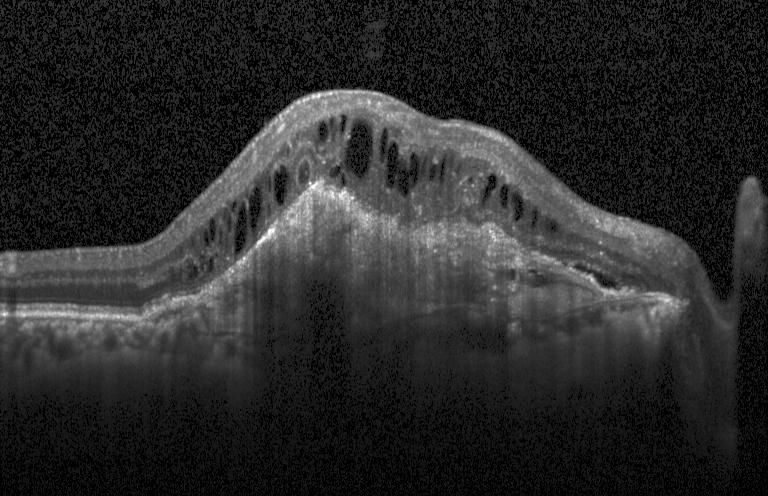
SD-OCT, instrument: Heidelberg Spectralis, retinal OCT B-scan
Diagnosis: a choroidal neovascular membrane.